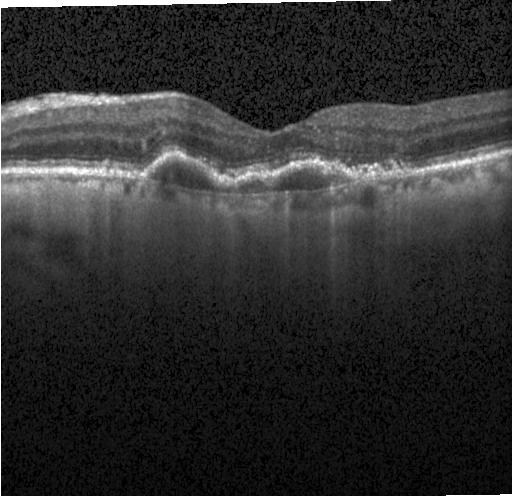 SD-OCT · retinal OCT cross-section · Heidelberg Spectralis OCT system · fovea-centered — This B-scan demonstrates a choroidal neovascular membrane.